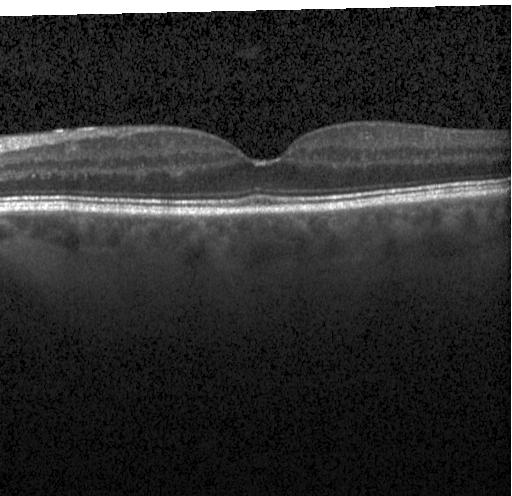

Optical coherence tomography scan
This B-scan demonstrates neither choroidal neovascularization, diabetic macular edema, nor drusen.